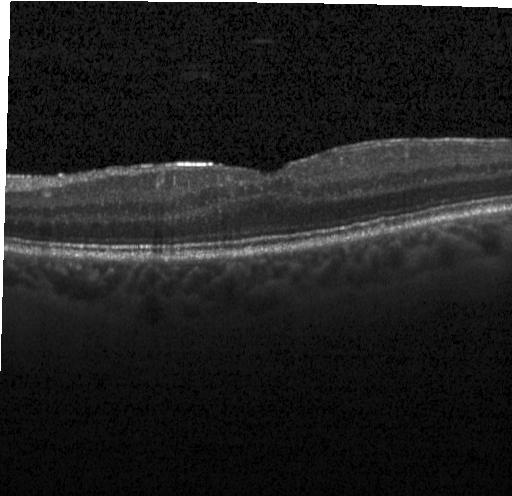

Impression: no evidence of choroidal neovascularization, diabetic macular edema, or drusen.